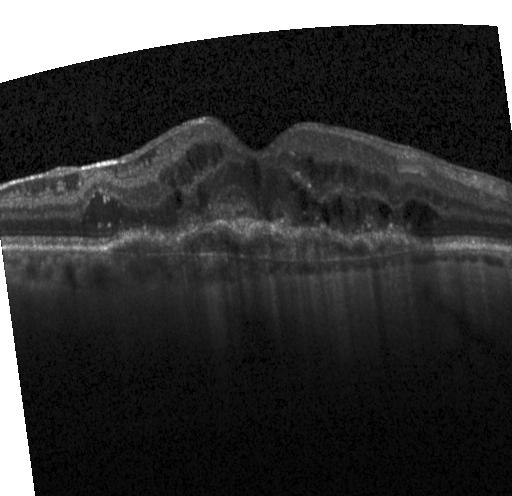 Diagnosis: a choroidal neovascular membrane.